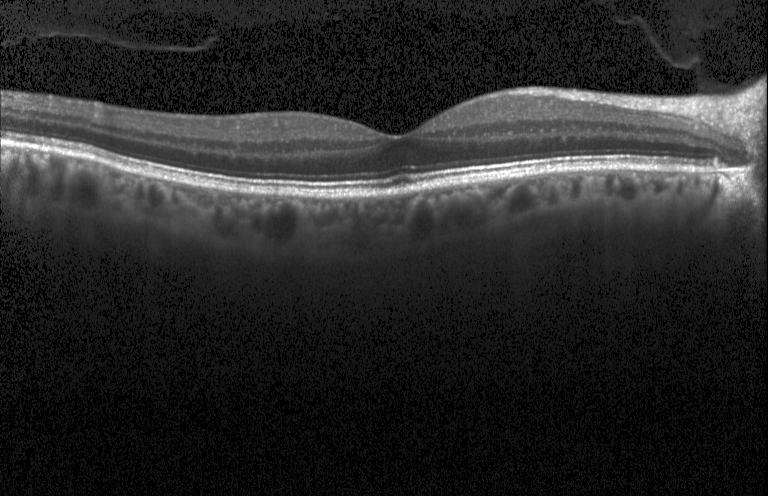

Heidelberg Spectralis. Spectral-domain OCT. Retinal OCT cross-section — Impression: no choroidal neovascularization, no diabetic macular edema, and no drusen.